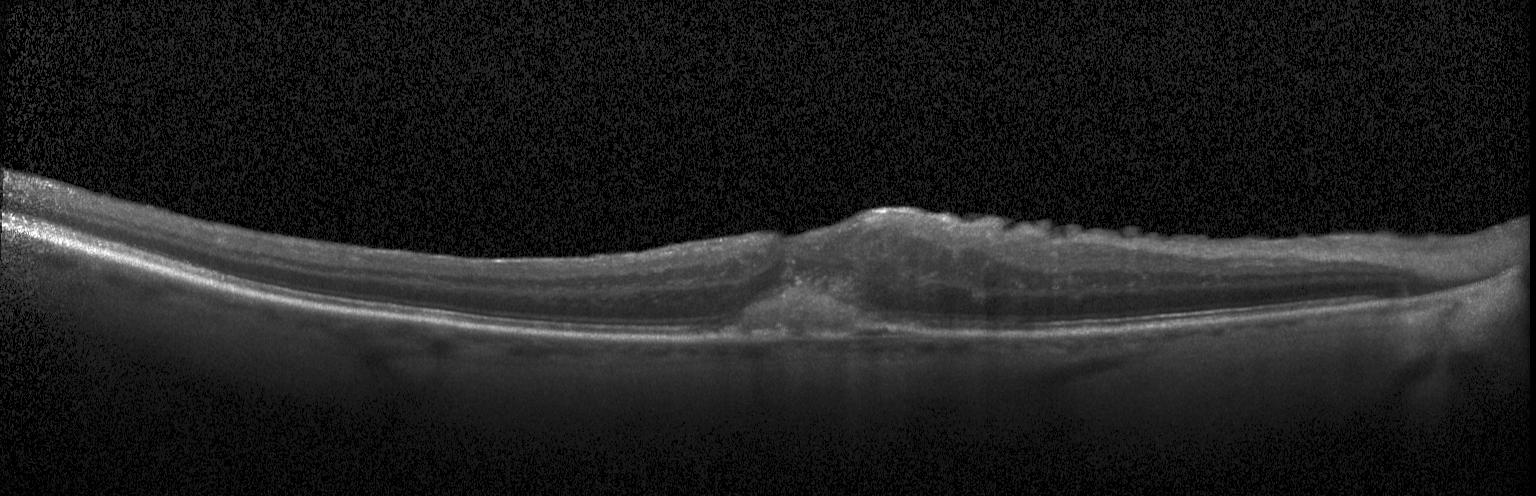
Finding: a choroidal neovascular membrane.